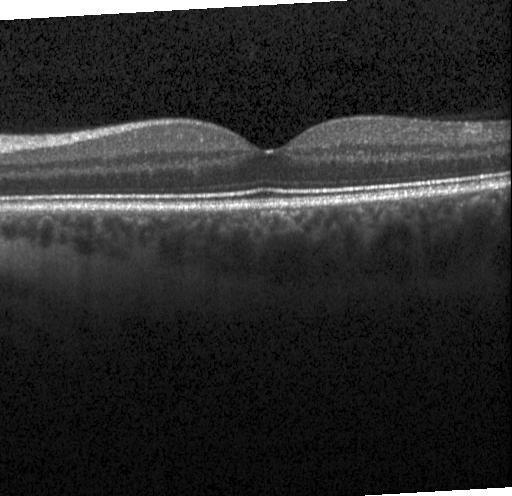
Spectral-domain optical coherence tomography, retinal OCT cross-section, Heidelberg Spectralis. Finding: neither CNV, DME, nor drusen.